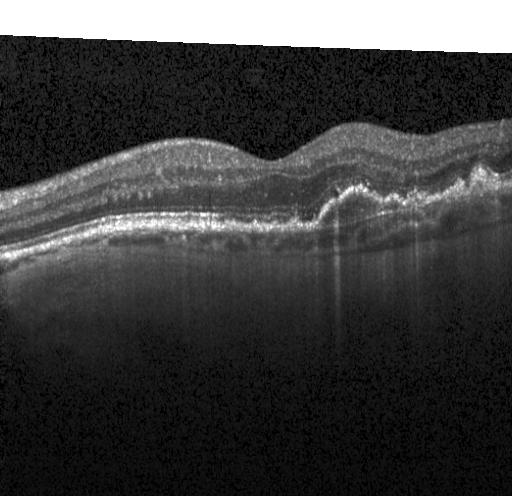
Optical coherence tomography B-scan; spectral-domain OCT
Assessment: CNV.